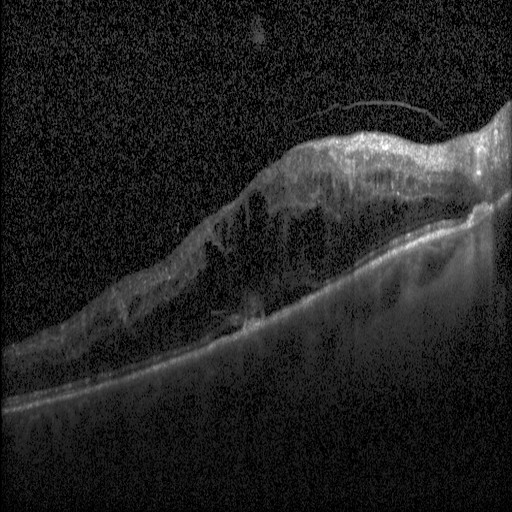

Impression: DME.